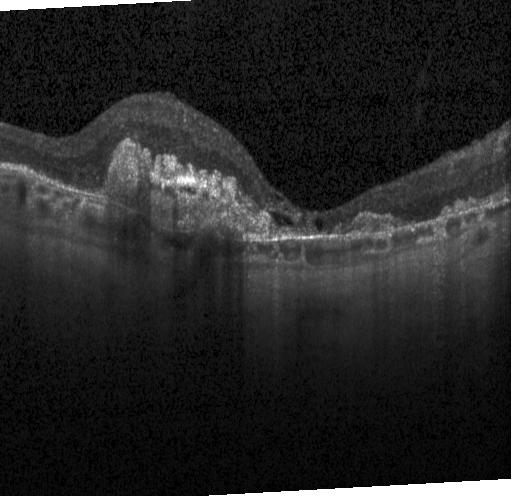

Retinal OCT B-scan; acquired on a Heidelberg Spectralis; SD-OCT. OCT finding: CNV.